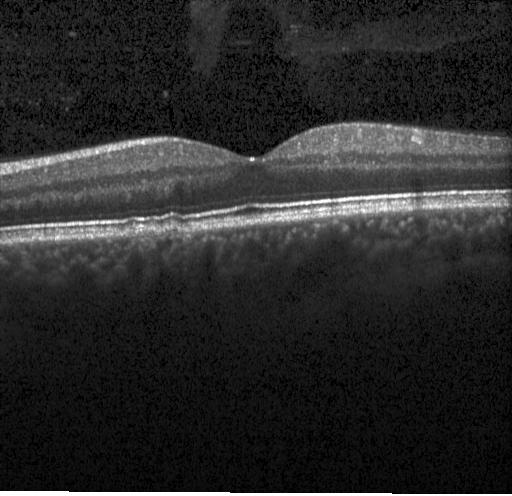

Optical coherence tomography scan.
This B-scan demonstrates sub-RPE drusenoid deposits.